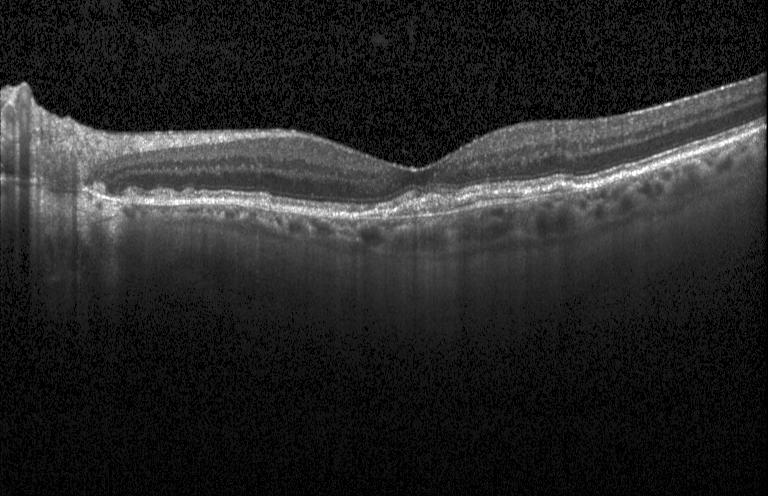 Finding: a choroidal neovascular membrane.